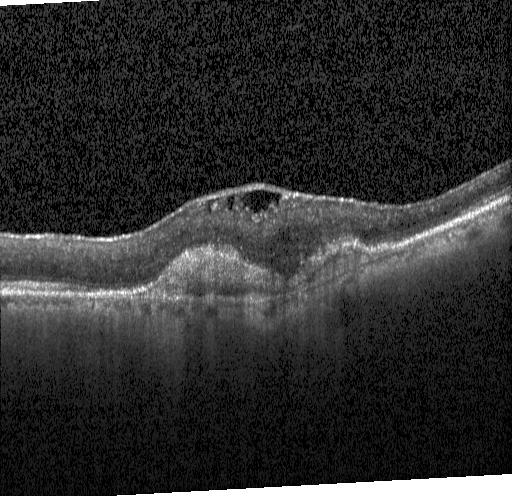 Acquired on a Heidelberg Spectralis · spectral-domain optical coherence tomography · OCT line scan. Impression: a choroidal neovascular membrane.